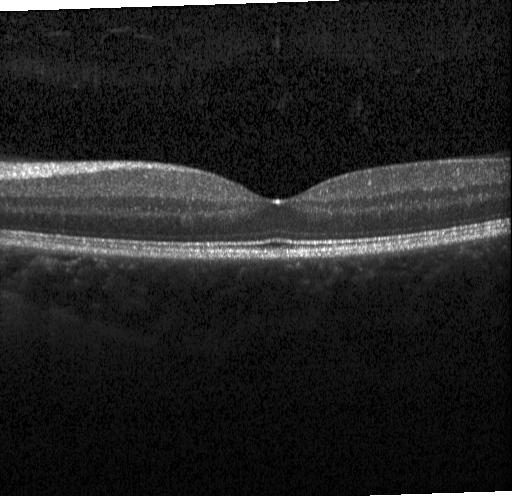

Spectral-domain optical coherence tomography · retinal OCT B-scan. Finding: no evidence of choroidal neovascularization, diabetic macular edema, or drusen.